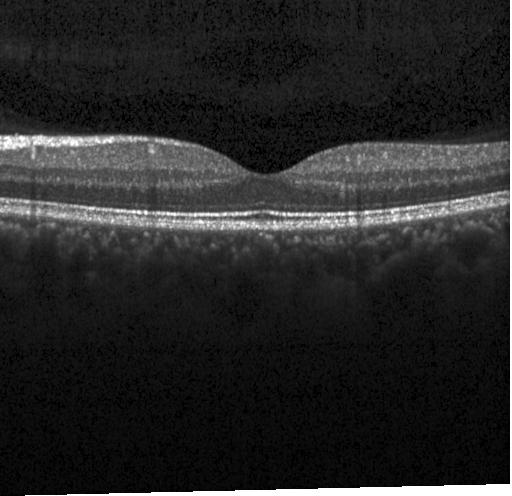
Retinal OCT cross-section. Macular OCT: neither choroidal neovascularization, diabetic macular edema, nor drusen.